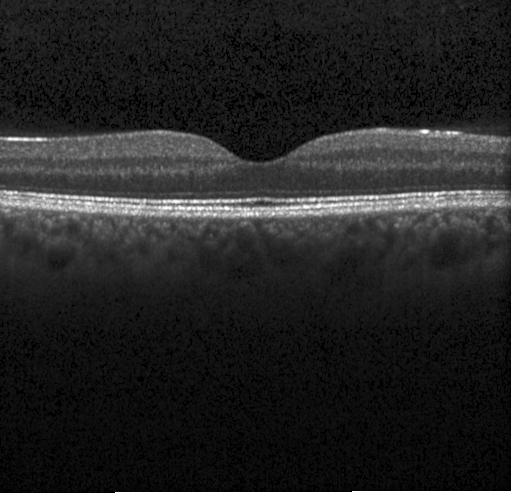

Dx: no evidence of choroidal neovascularization, diabetic macular edema, or drusen.